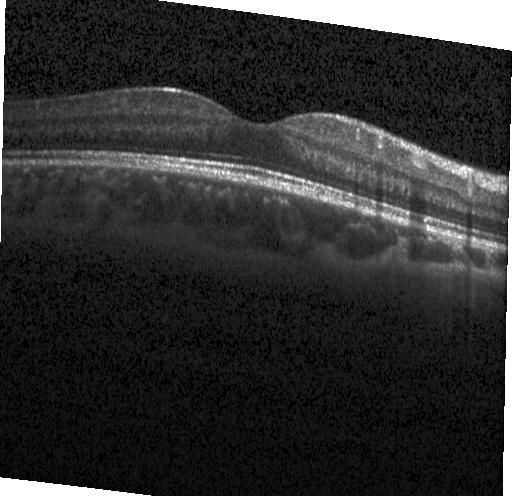

Instrument: Heidelberg Spectralis; spectral-domain optical coherence tomography; OCT line scan.
Macular OCT: no choroidal neovascularization, no diabetic macular edema, and no drusen.